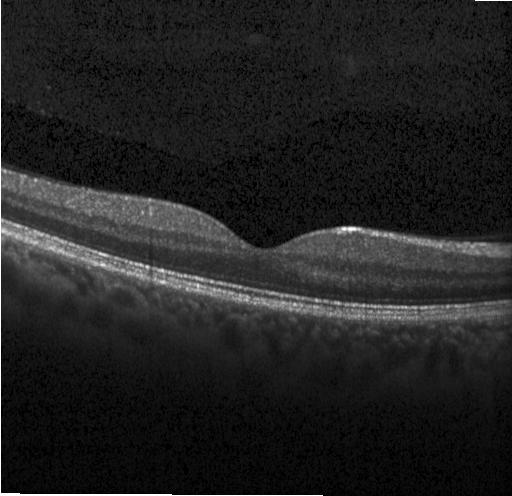
Retinal OCT cross-section. The scan shows no choroidal neovascularization, no diabetic macular edema, and no drusen.